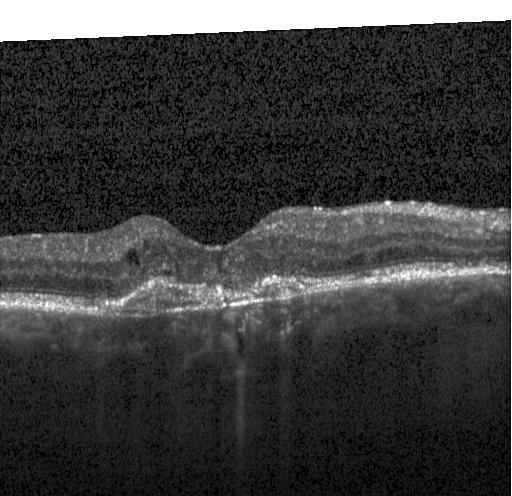 Retinal OCT cross-section.
Dx: choroidal neovascularization (CNV).